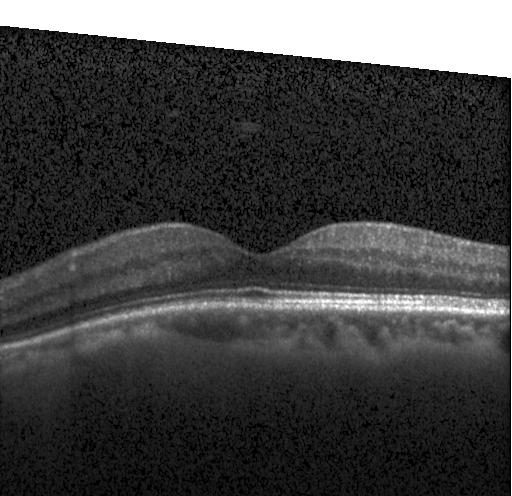

SD-OCT. Retinal OCT cross-section — Neither CNV, DME, nor drusen.